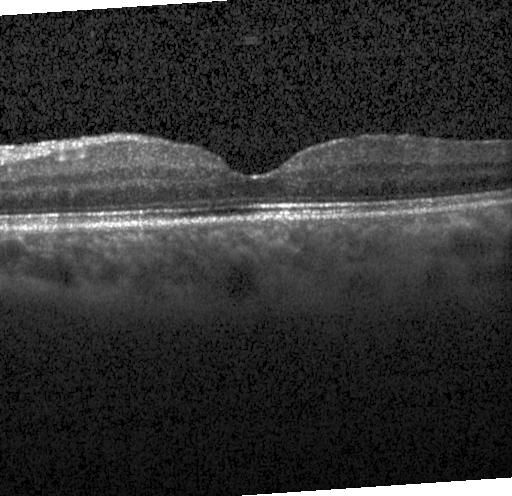 Heidelberg Spectralis; centered on the fovea; retinal OCT cross-section; SD-OCT.
Diagnosis: neither choroidal neovascularization, diabetic macular edema, nor drusen.